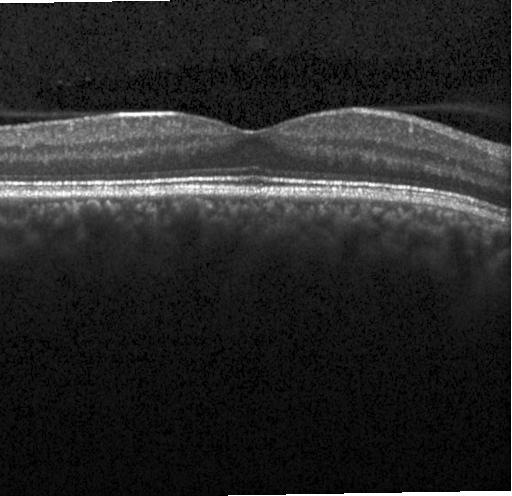

Impression: no evidence of choroidal neovascularization, diabetic macular edema, or drusen.